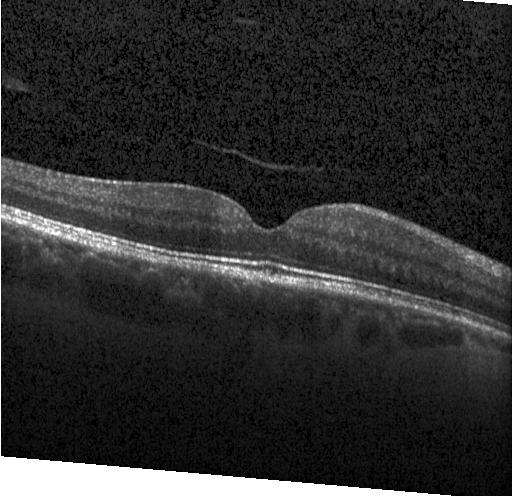

Diagnosis: no choroidal neovascularization, no diabetic macular edema, and no drusen.